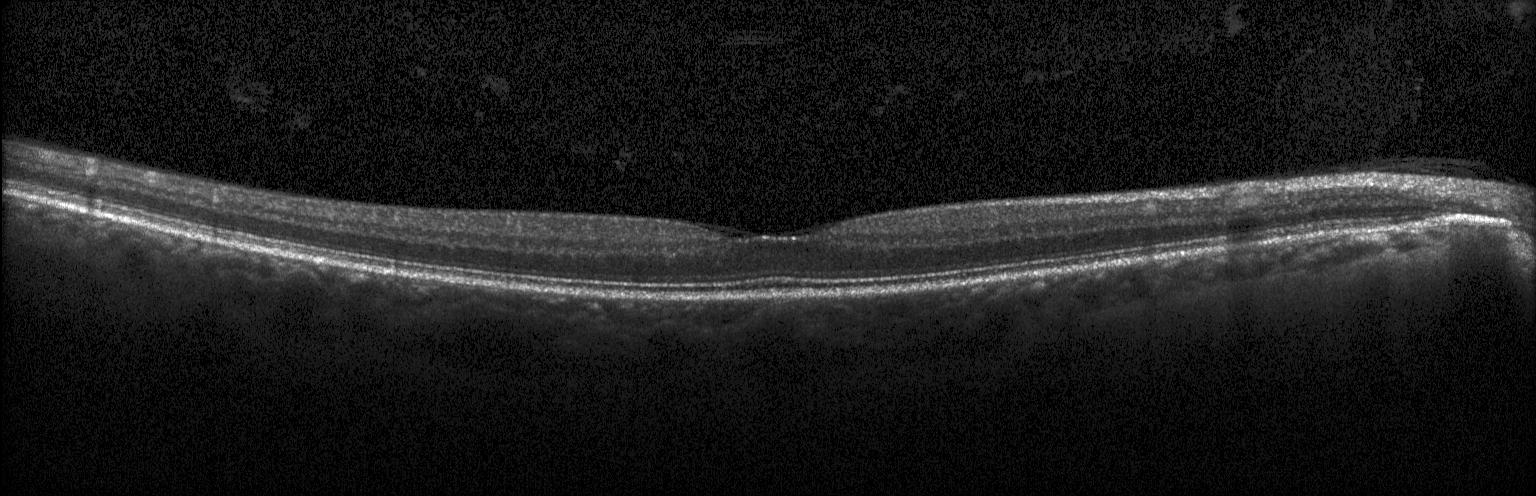
OCT B-scan
The scan shows no choroidal neovascularization, no diabetic macular edema, and no drusen.